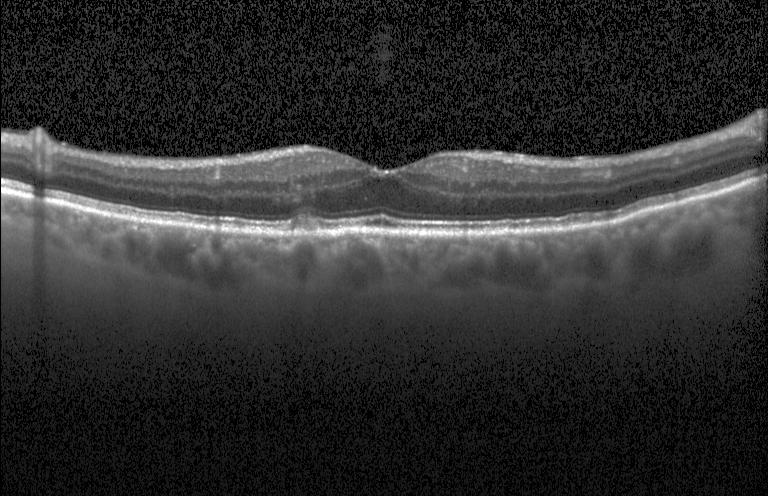 Heidelberg Spectralis; OCT line scan; spectral-domain optical coherence tomography; macular scan — Assessment: multiple drusen.